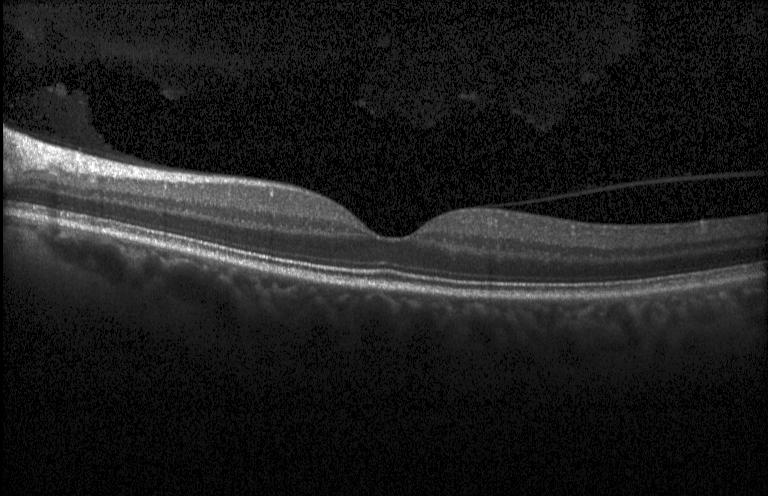
The scan shows no CNV, no DME, and no drusen.